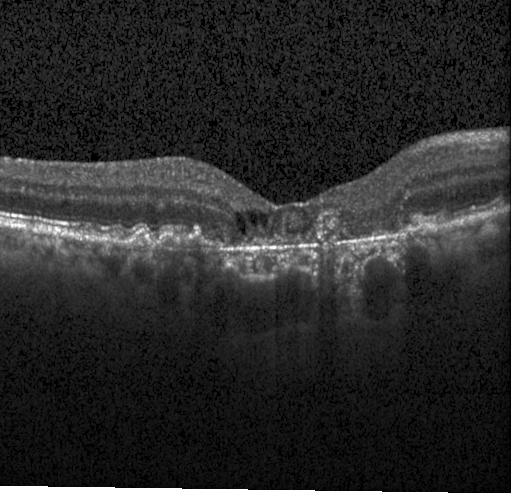

Acquired on a Heidelberg Spectralis · spectral-domain optical coherence tomography · centered on the fovea · retinal OCT B-scan — The scan shows a choroidal neovascular membrane.